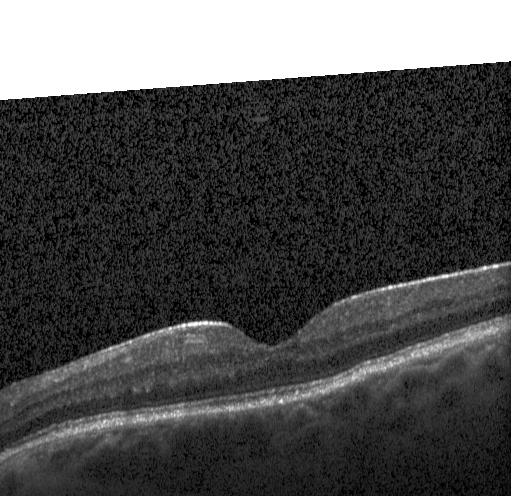
Impression: no choroidal neovascularization, no diabetic macular edema, and no drusen.